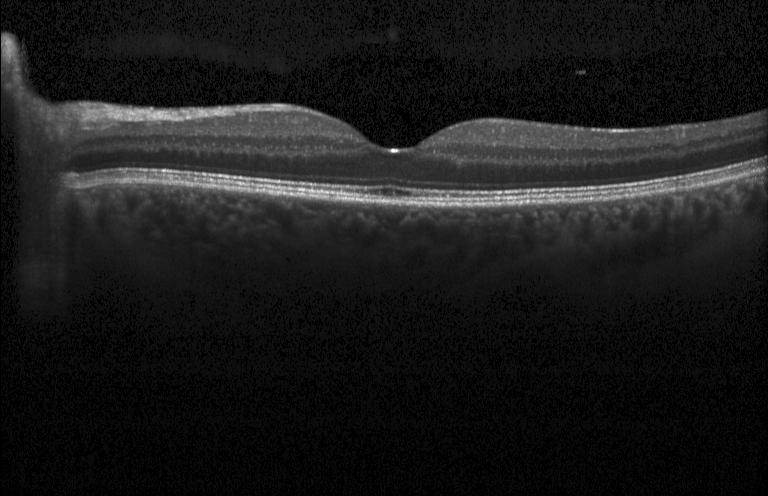 Spectral-domain OCT · centered on the fovea · retinal OCT cross-section.
OCT finding: no CNV, no DME, and no drusen.